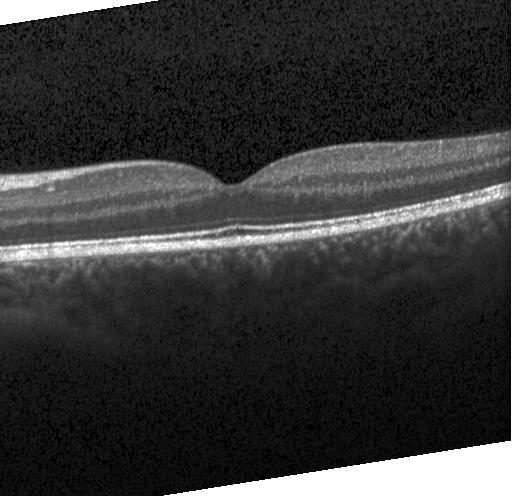 Centered on the fovea, optical coherence tomography B-scan
Diagnosis: no choroidal neovascularization, no diabetic macular edema, and no drusen.